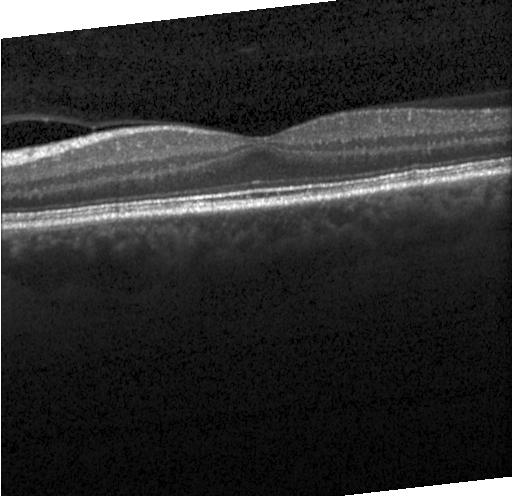
Macular OCT demonstrating neither CNV, DME, nor drusen.